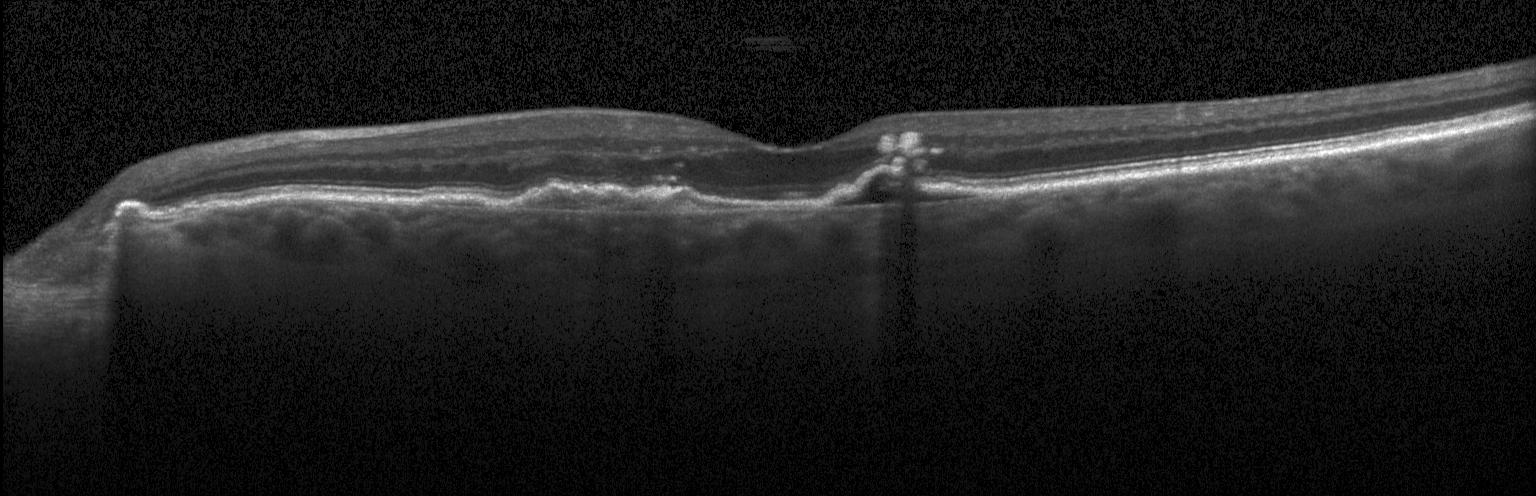

Optical coherence tomography B-scan — OCT finding: a choroidal neovascular membrane.